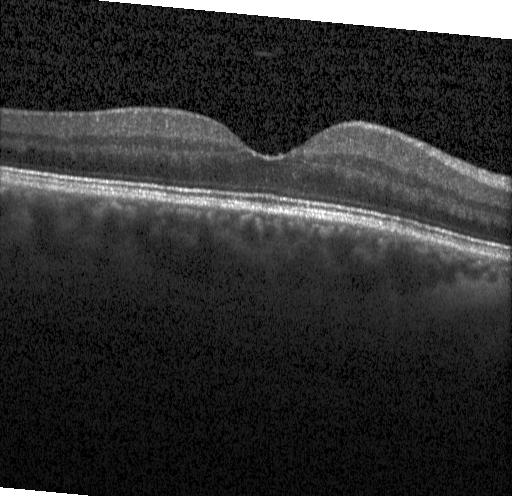
OCT line scan · instrument: Heidelberg Spectralis · macular scan — This B-scan demonstrates neither choroidal neovascularization, diabetic macular edema, nor drusen.